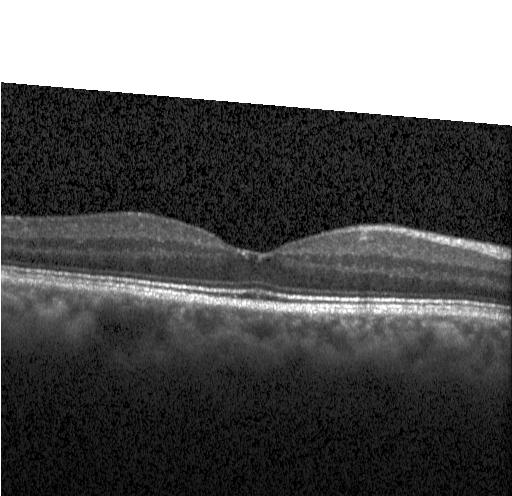

Impression: no choroidal neovascularization, no diabetic macular edema, and no drusen.